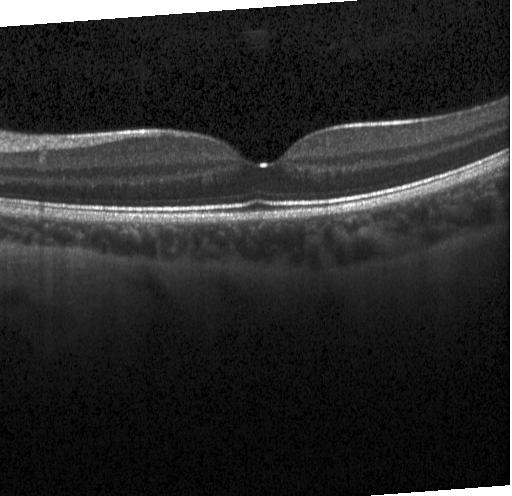
OCT B-scan; SD-OCT. No evidence of choroidal neovascularization, diabetic macular edema, or drusen.